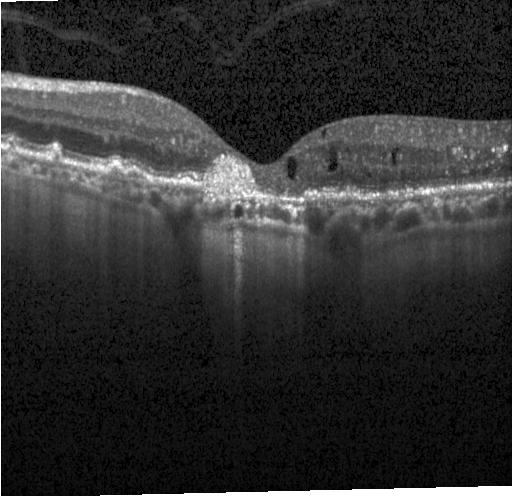 OCT line scan. Macular scan. Heidelberg Spectralis OCT system. Spectral-domain optical coherence tomography. Diagnosis: CNV.